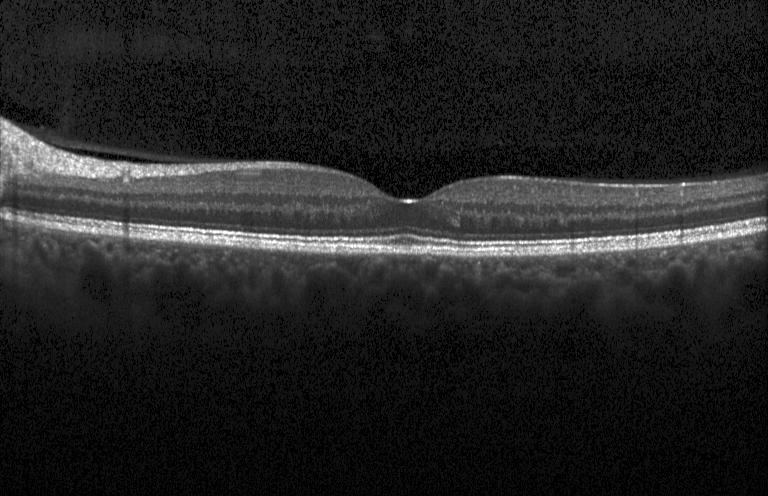
Optical coherence tomography scan — Impression: no choroidal neovascularization, no diabetic macular edema, and no drusen.